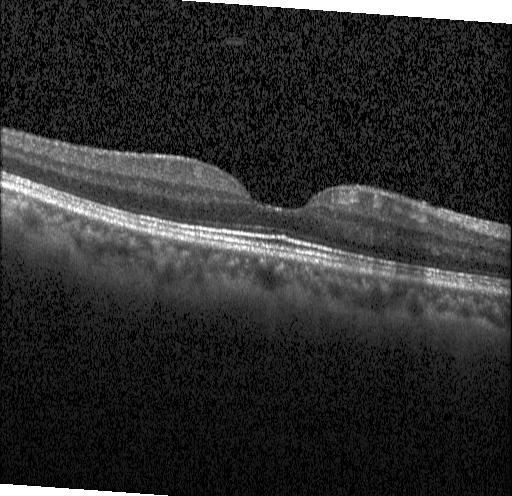 Optical coherence tomography scan, fovea-centered.
Finding: no choroidal neovascularization, no diabetic macular edema, and no drusen.